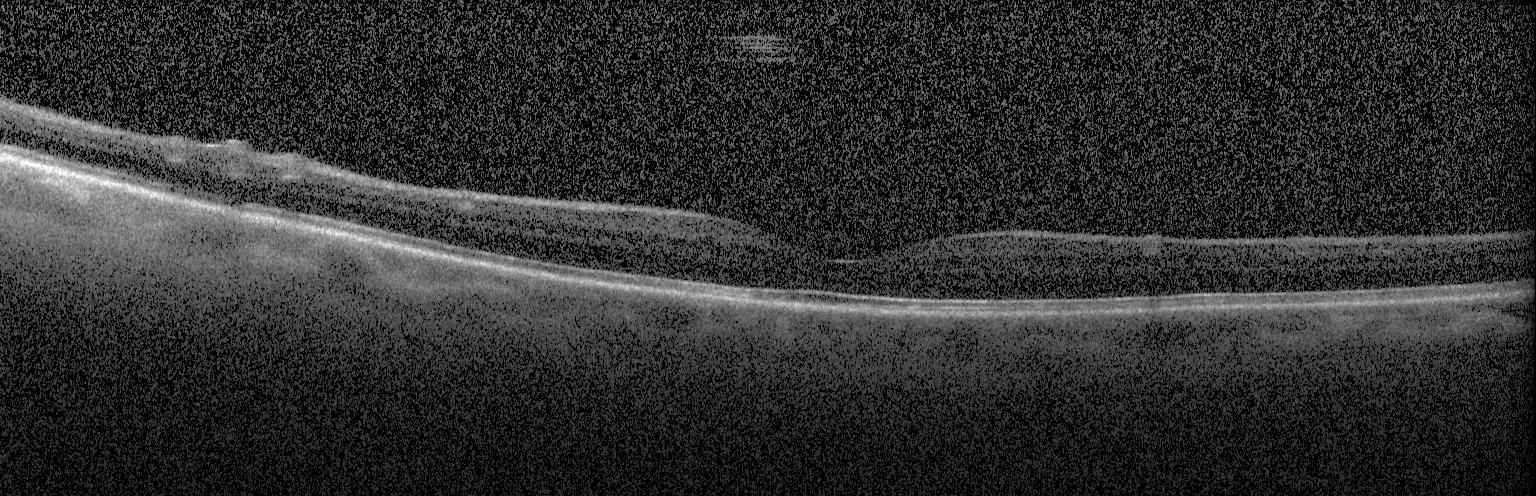

Macular scan; retinal OCT B-scan; Heidelberg Spectralis
The scan shows neither choroidal neovascularization, diabetic macular edema, nor drusen.